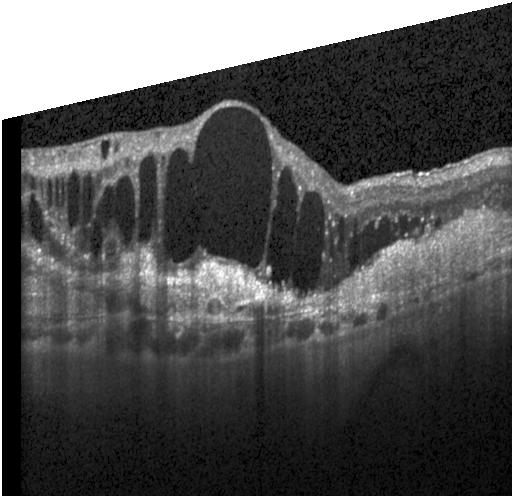

Centered on the fovea; instrument: Heidelberg Spectralis; OCT line scan — OCT finding: choroidal neovascularization.